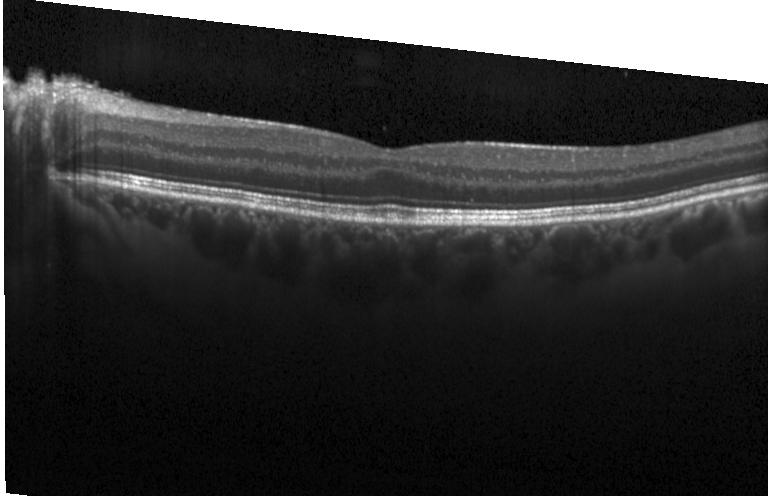 Spectral-domain OCT B-scan: no evidence of choroidal neovascularization, diabetic macular edema, or drusen.